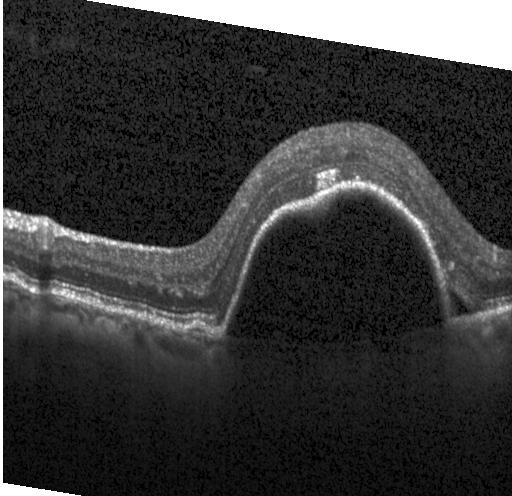 OCT line scan, Heidelberg Spectralis OCT system
Assessment: a choroidal neovascular membrane.